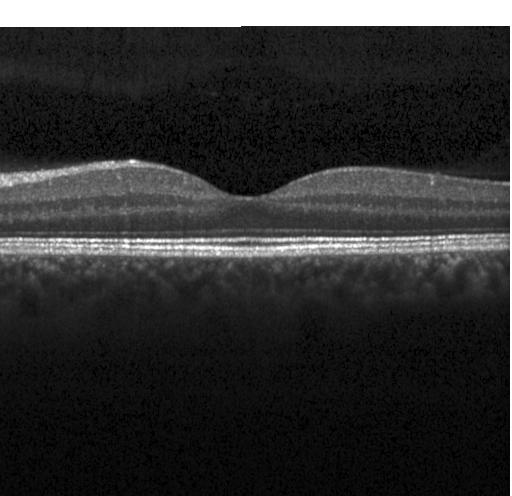 Impression: no evidence of CNV, DME, or drusen.